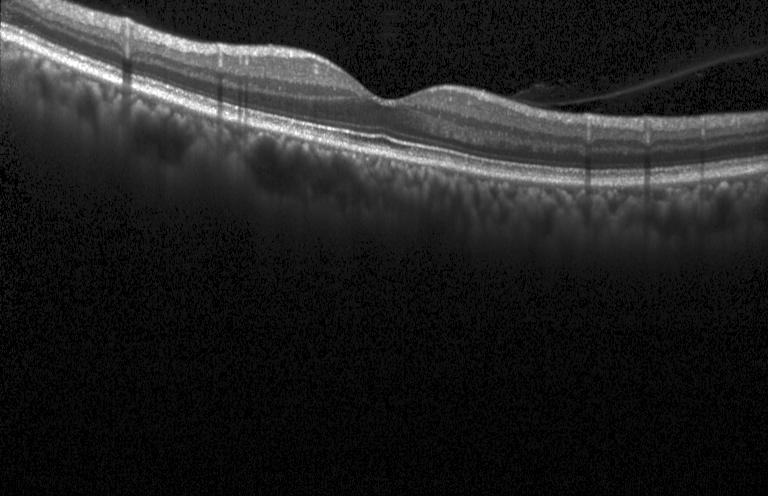

Horizontal scan through the fovea · OCT B-scan · SD-OCT. The scan shows no choroidal neovascularization, no diabetic macular edema, and no drusen.